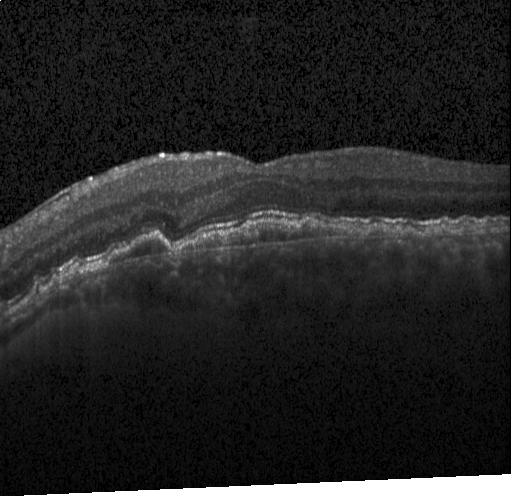 Acquired on a Heidelberg Spectralis. OCT line scan.
The scan shows a choroidal neovascular membrane.